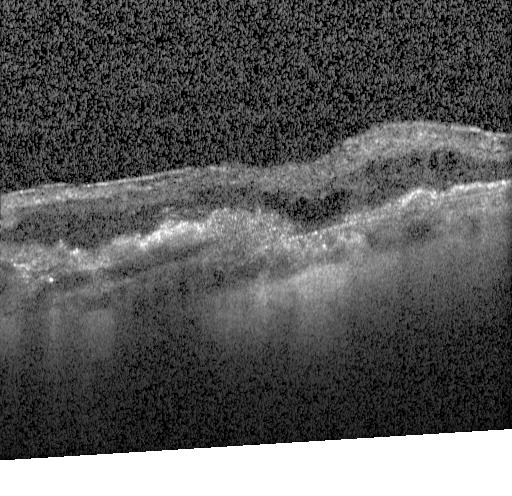
Horizontal scan through the fovea. Spectral-domain OCT. Instrument: Heidelberg Spectralis. OCT B-scan
Assessment: a choroidal neovascular membrane.